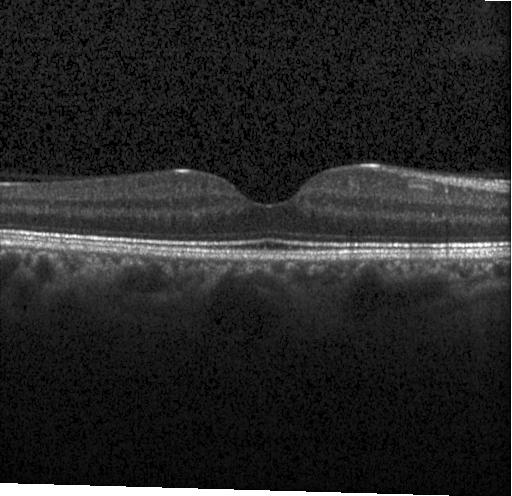
Retinal OCT B-scan, spectral-domain OCT — Diagnosis: no choroidal neovascularization, diabetic macular edema, or drusen.